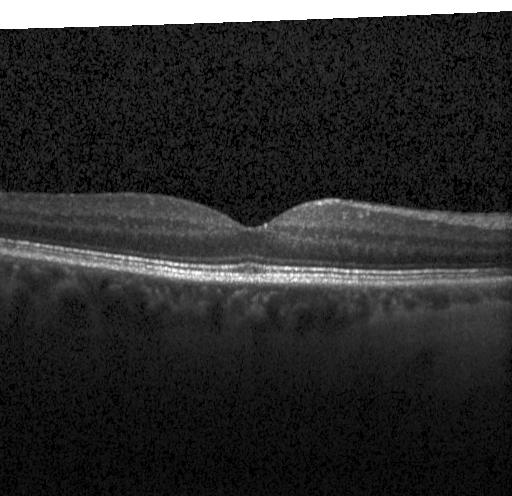

Impression: no choroidal neovascularization, diabetic macular edema, or drusen.